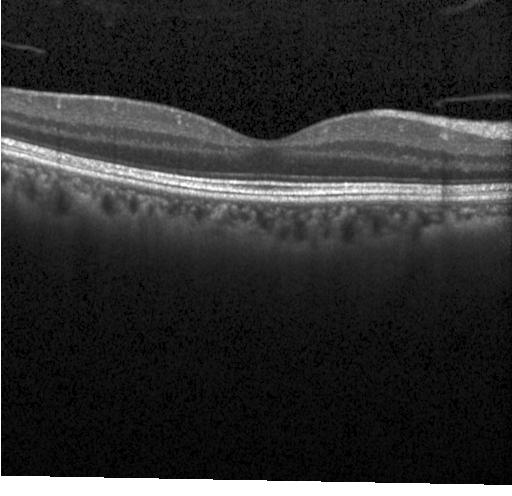

OCT scan showing no choroidal neovascularization, no diabetic macular edema, and no drusen.